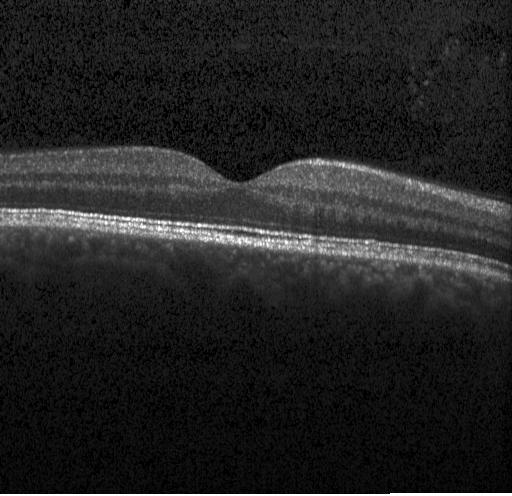 Retinal OCT cross-section. Horizontal scan through the fovea. Heidelberg Spectralis OCT system.
No evidence of choroidal neovascularization, diabetic macular edema, or drusen.